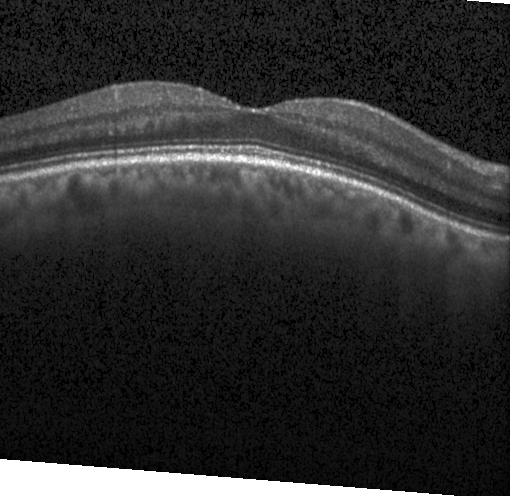

Impression: neither choroidal neovascularization, diabetic macular edema, nor drusen.